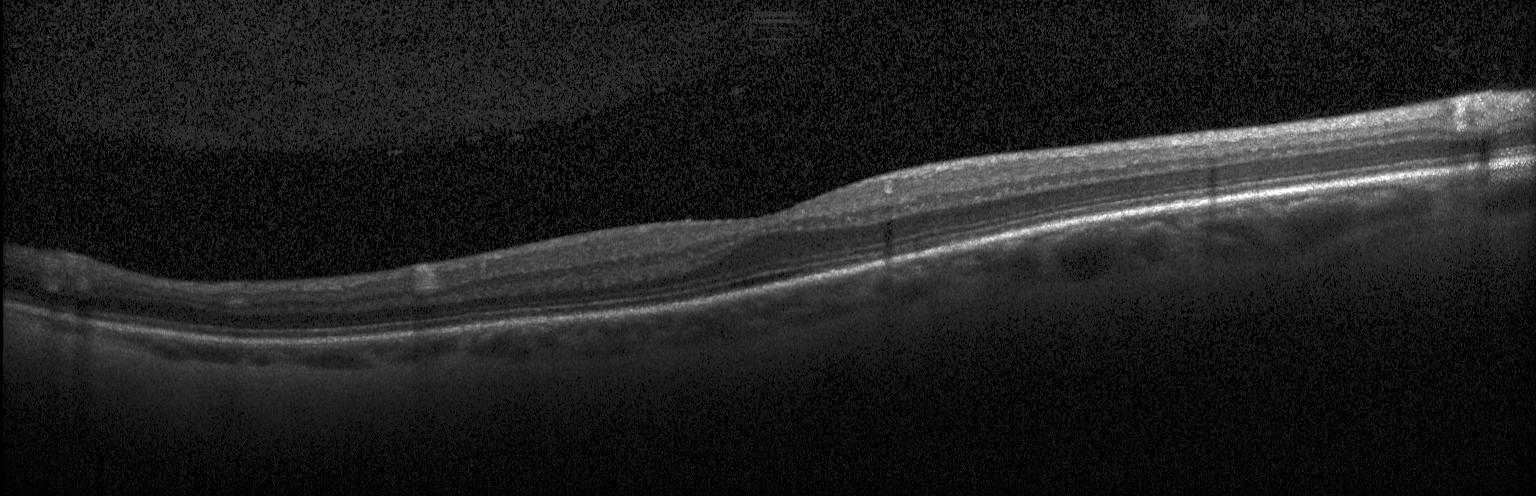
Finding: no choroidal neovascularization, diabetic macular edema, or drusen.